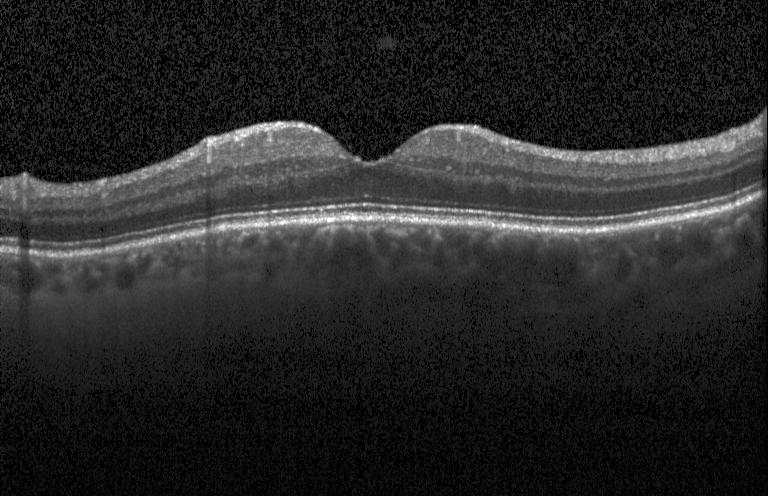

Macular OCT: no choroidal neovascularization, diabetic macular edema, or drusen.